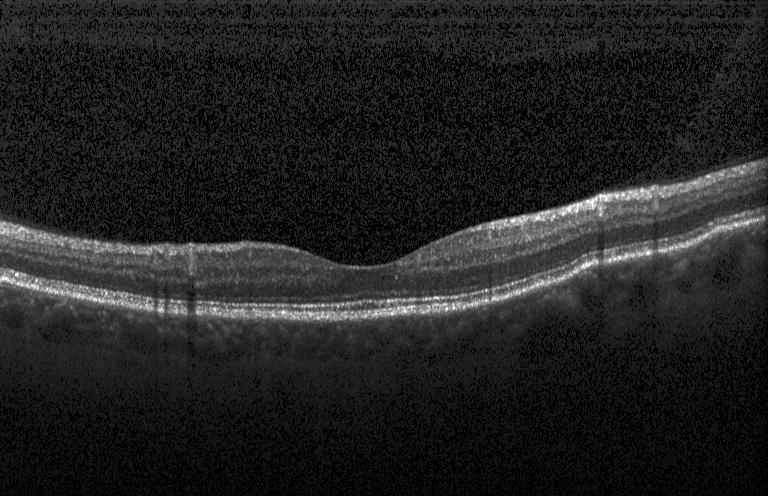

Centered on the fovea. Spectral-domain optical coherence tomography. Heidelberg Spectralis OCT system. OCT line scan — Diagnosis: neither choroidal neovascularization, diabetic macular edema, nor drusen.